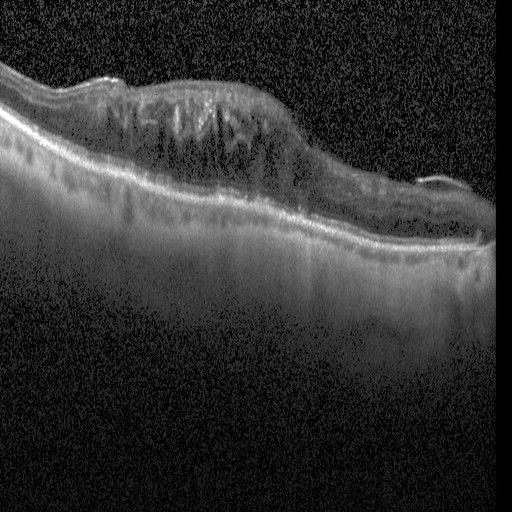 Through the macula, SD-OCT, OCT B-scan, Heidelberg Spectralis OCT system
Impression: diabetic macular edema (DME).